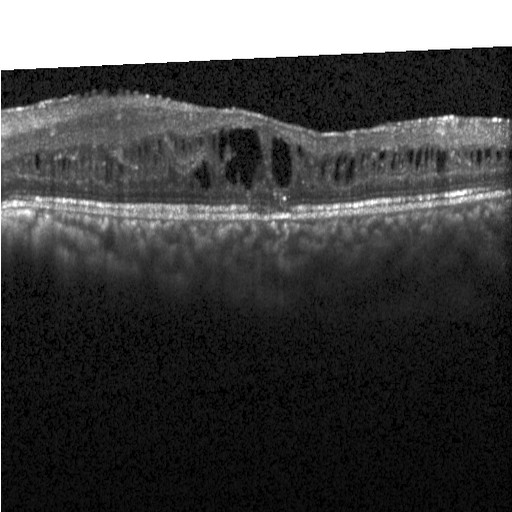

OCT line scan. Horizontal scan through the fovea. Acquired on a Heidelberg Spectralis. Spectral-domain OCT.
This B-scan demonstrates diabetic macular edema.